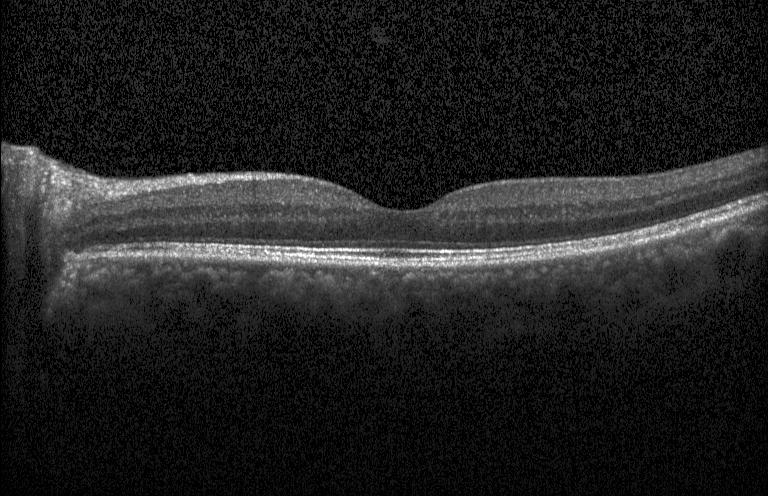

Optical coherence tomography scan; SD-OCT; instrument: Heidelberg Spectralis. Dx: no choroidal neovascularization, diabetic macular edema, or drusen.